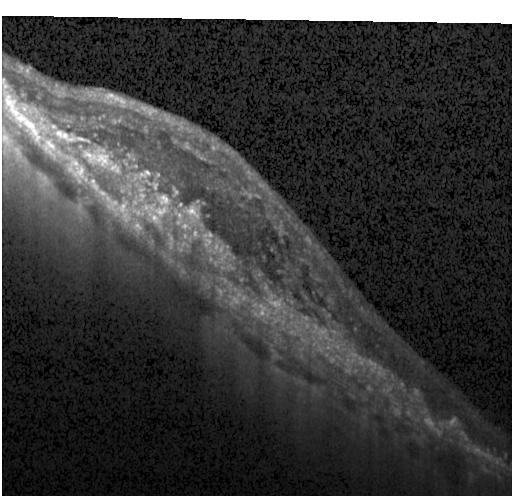

Optical coherence tomography scan, spectral-domain OCT, acquired on a Heidelberg Spectralis, through the macula
Impression: a choroidal neovascular membrane.